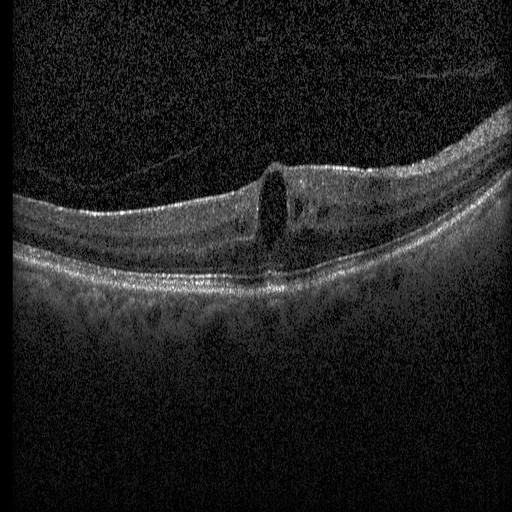
Through the macula; Heidelberg Spectralis OCT system; retinal OCT B-scan — OCT finding: diabetic macular edema (DME).